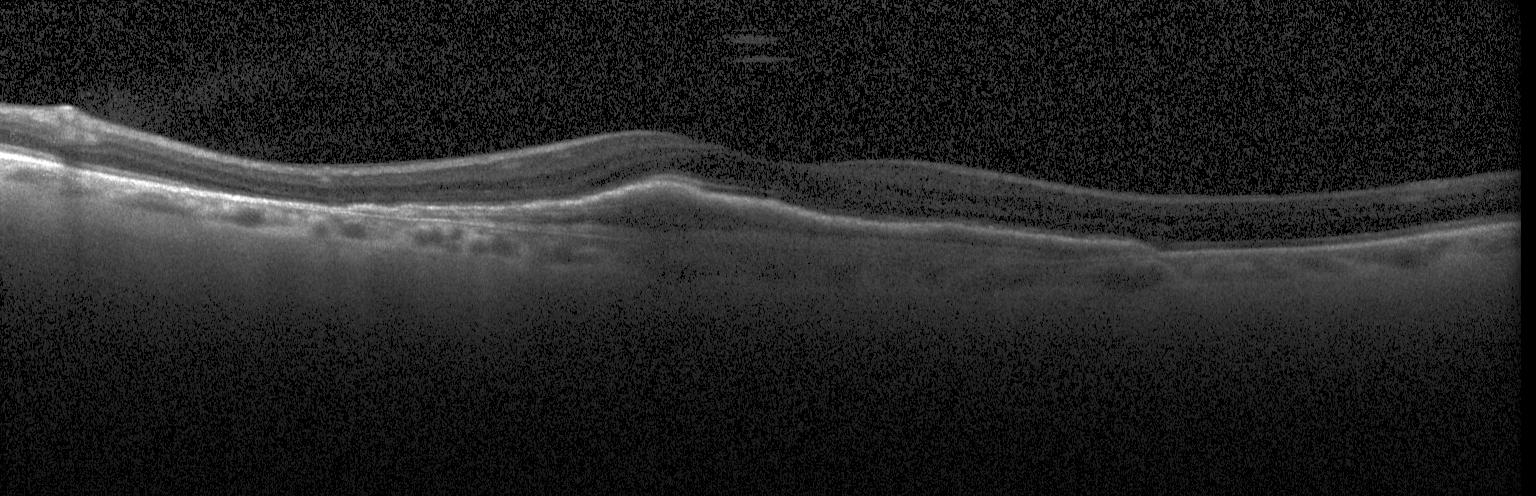
Impression: choroidal neovascularization (CNV).